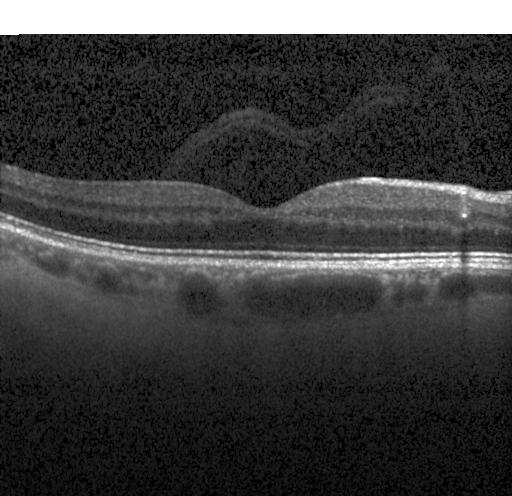 Dx: neither CNV, DME, nor drusen.